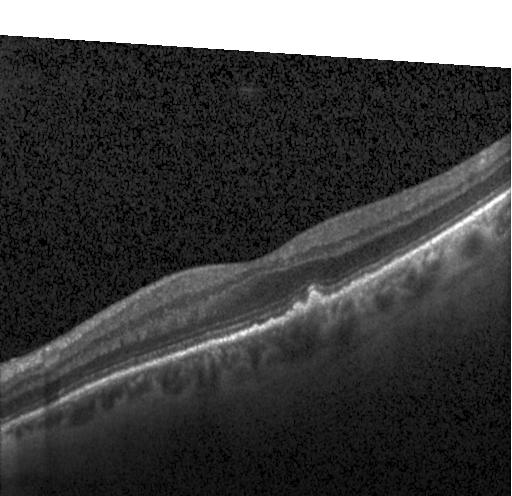

OCT B-scan — Finding: multiple drusen.